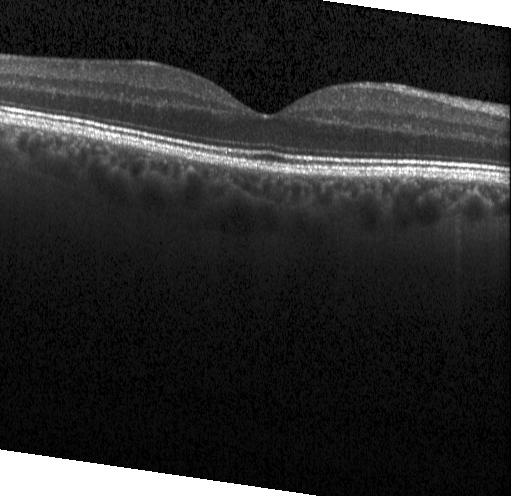

Optical coherence tomography B-scan. Spectral-domain OCT. Centered on the fovea
Assessment: no choroidal neovascularization, no diabetic macular edema, and no drusen.